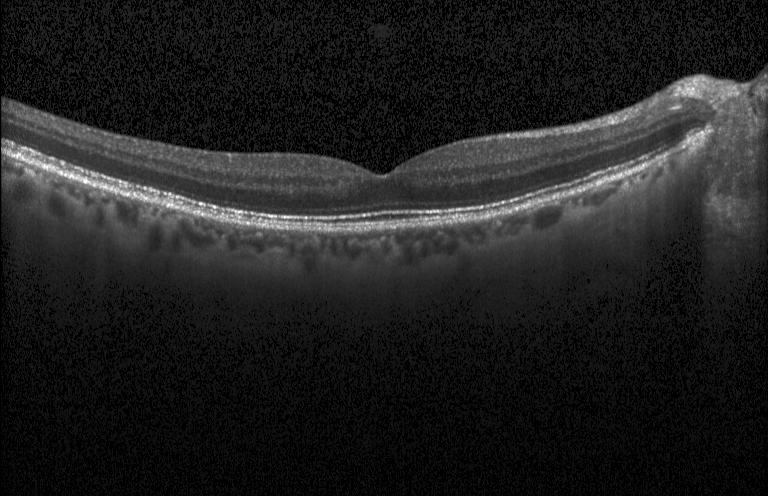

Diagnosis: no evidence of choroidal neovascularization, diabetic macular edema, or drusen.